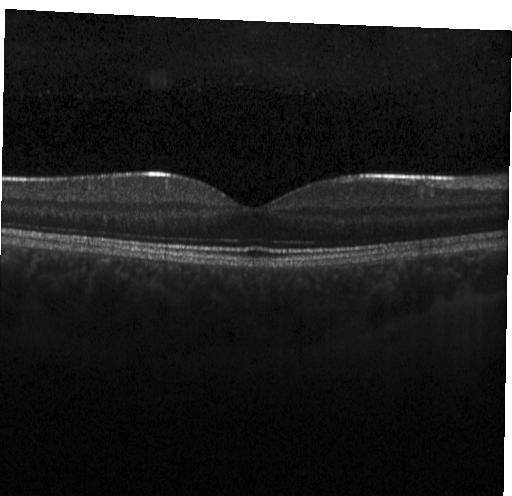
Acquired on a Heidelberg Spectralis; retinal OCT B-scan; fovea-centered — Diagnosis: no choroidal neovascularization, no diabetic macular edema, and no drusen.